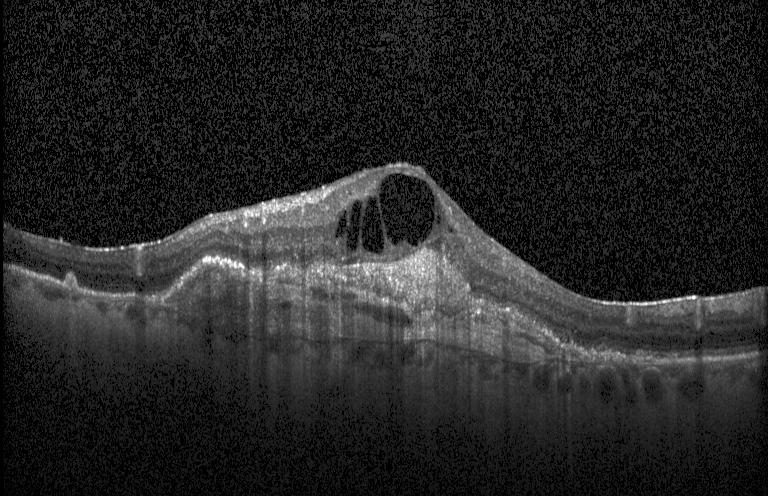

Impression: a choroidal neovascular membrane.